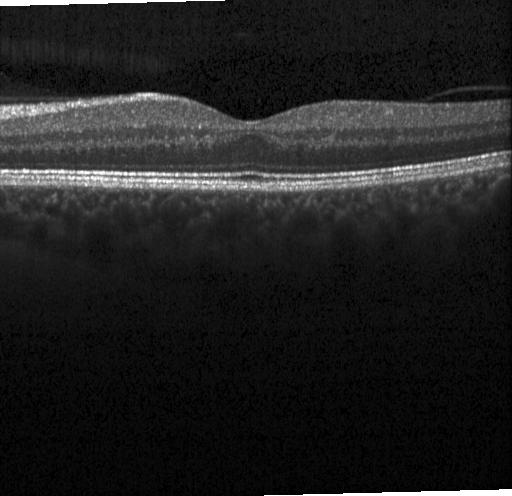
Heidelberg Spectralis; retinal OCT cross-section.
Diagnosis: no choroidal neovascularization, diabetic macular edema, or drusen.